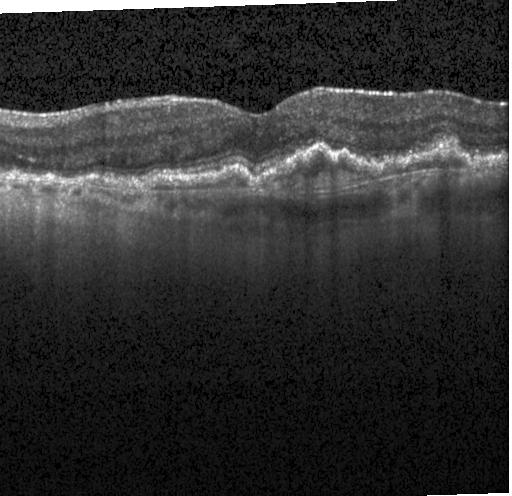 Acquired on a Heidelberg Spectralis. Through the macula. Retinal OCT B-scan. Spectral-domain optical coherence tomography
Finding: CNV.